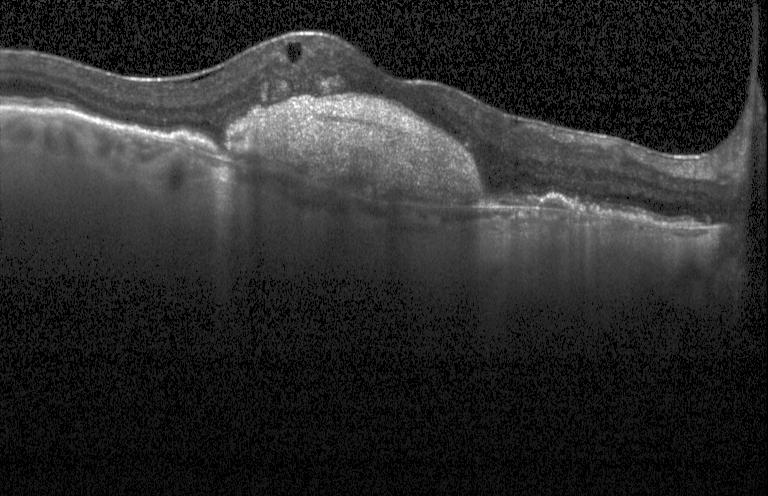
Heidelberg Spectralis OCT system. SD-OCT. Horizontal scan through the fovea. Optical coherence tomography B-scan. Dx: choroidal neovascularization.